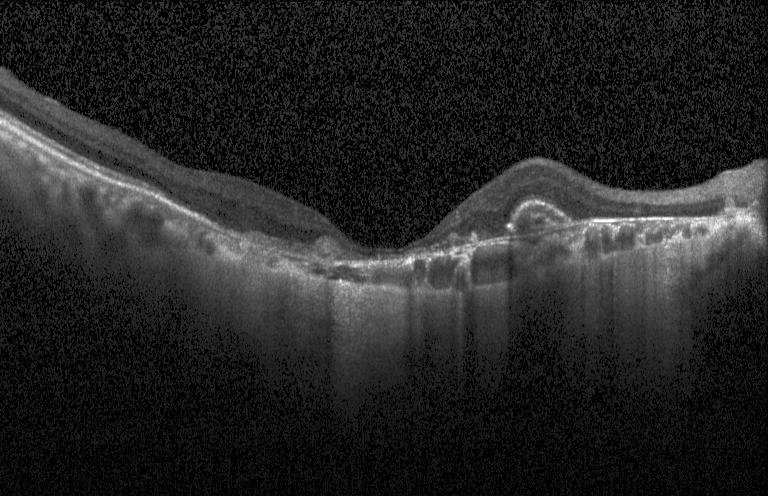

Retinal OCT cross-section. Heidelberg Spectralis.
Impression: a choroidal neovascular membrane.